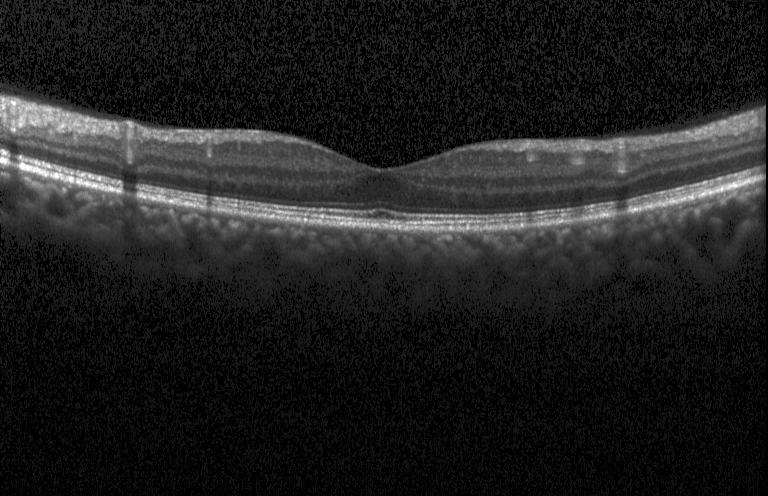 Retinal OCT B-scan; instrument: Heidelberg Spectralis; fovea-centered.
This B-scan demonstrates neither choroidal neovascularization, diabetic macular edema, nor drusen.